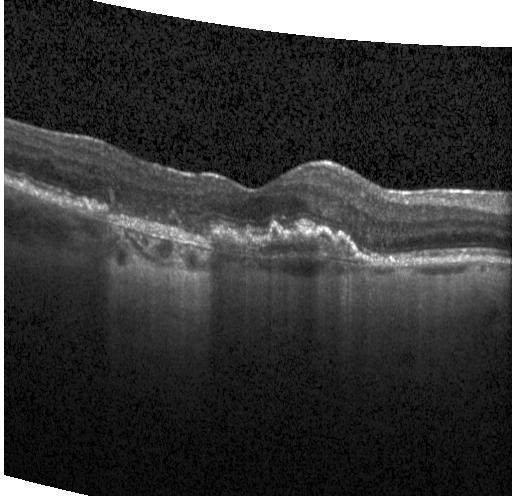

Diagnosis: a choroidal neovascular membrane.